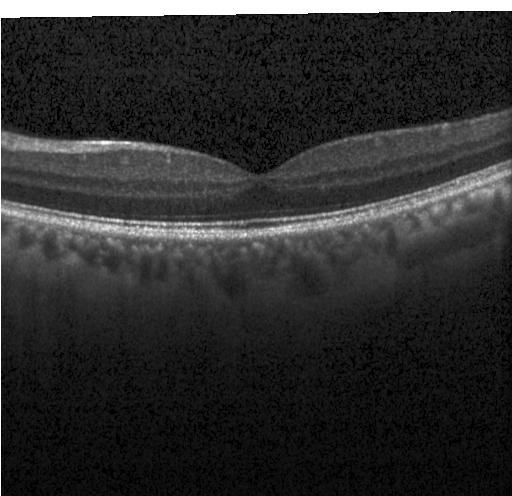
Spectral-domain OCT B-scan: no choroidal neovascularization, no diabetic macular edema, and no drusen.